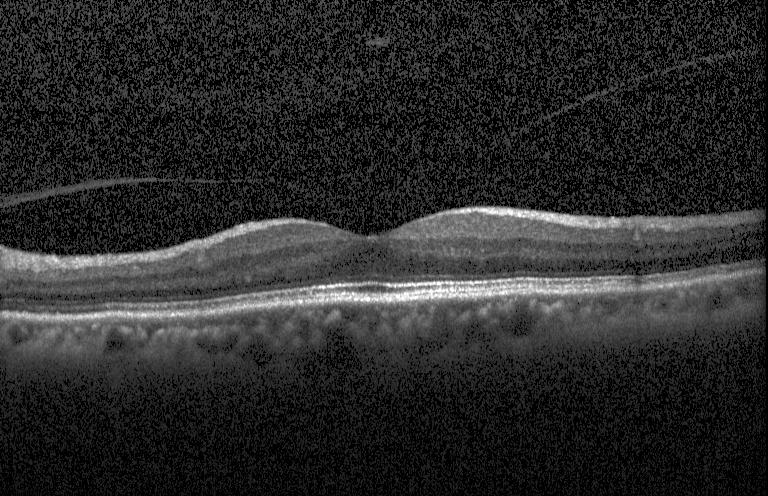
Diagnosis: neither CNV, DME, nor drusen.